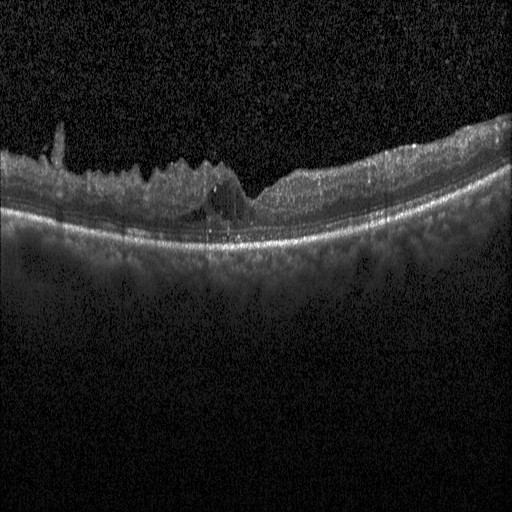 Finding: diabetic macular edema.